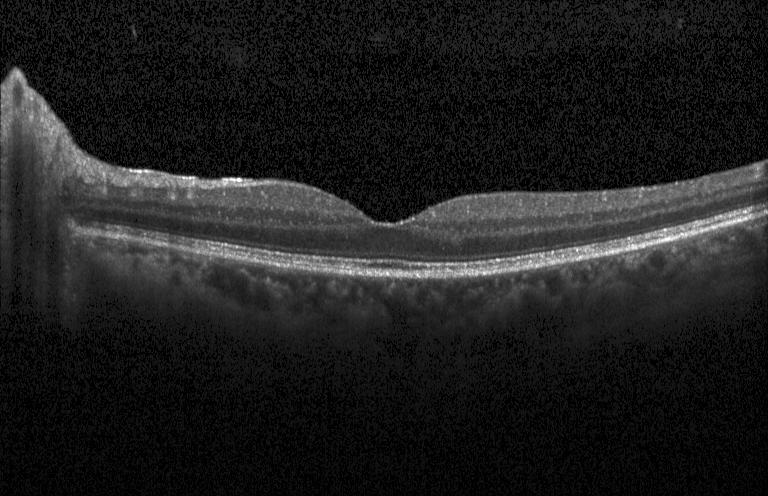

Heidelberg Spectralis, spectral-domain OCT, retinal OCT B-scan
This B-scan demonstrates no CNV, no DME, and no drusen.